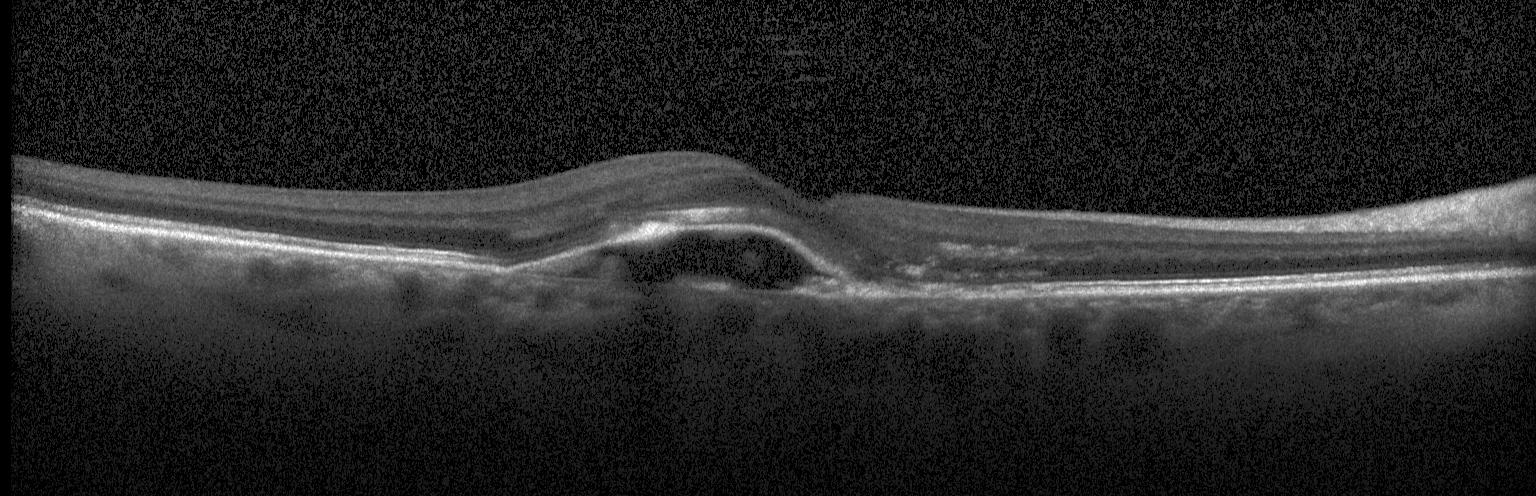 Spectral-domain OCT B-scan: choroidal neovascularization.